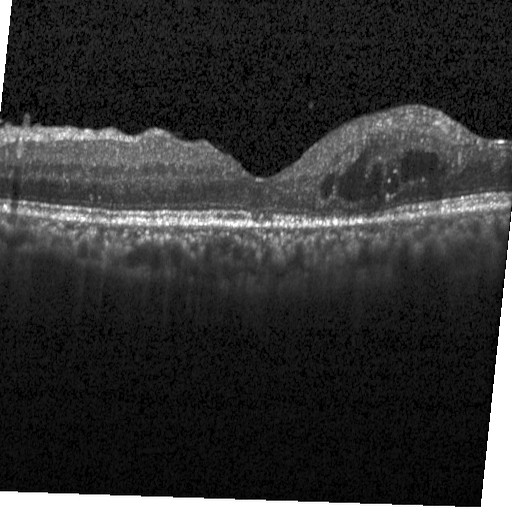
Spectral-domain OCT, centered on the fovea, retinal OCT cross-section, Heidelberg Spectralis — Dx: DME.